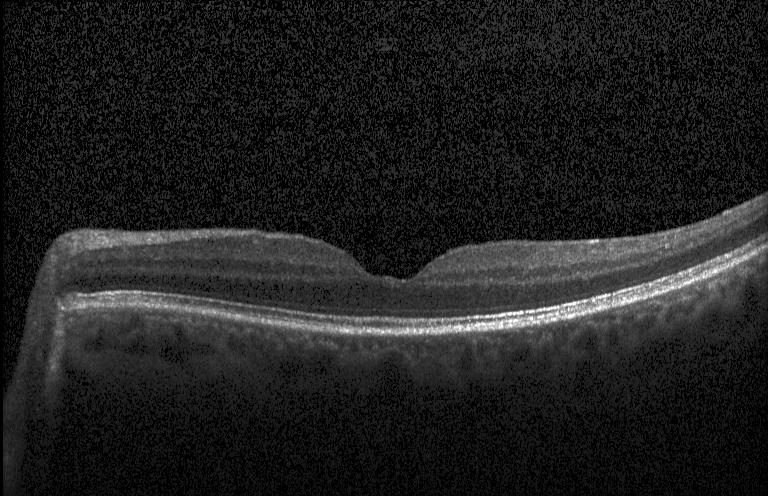

Spectral-domain OCT B-scan: no evidence of choroidal neovascularization, diabetic macular edema, or drusen.